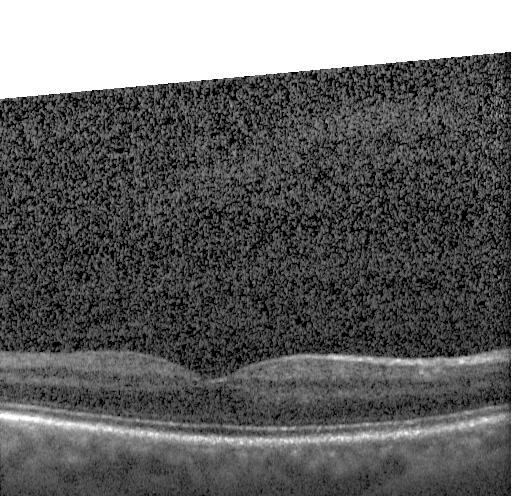
Instrument: Heidelberg Spectralis. OCT line scan
No choroidal neovascularization, no diabetic macular edema, and no drusen.